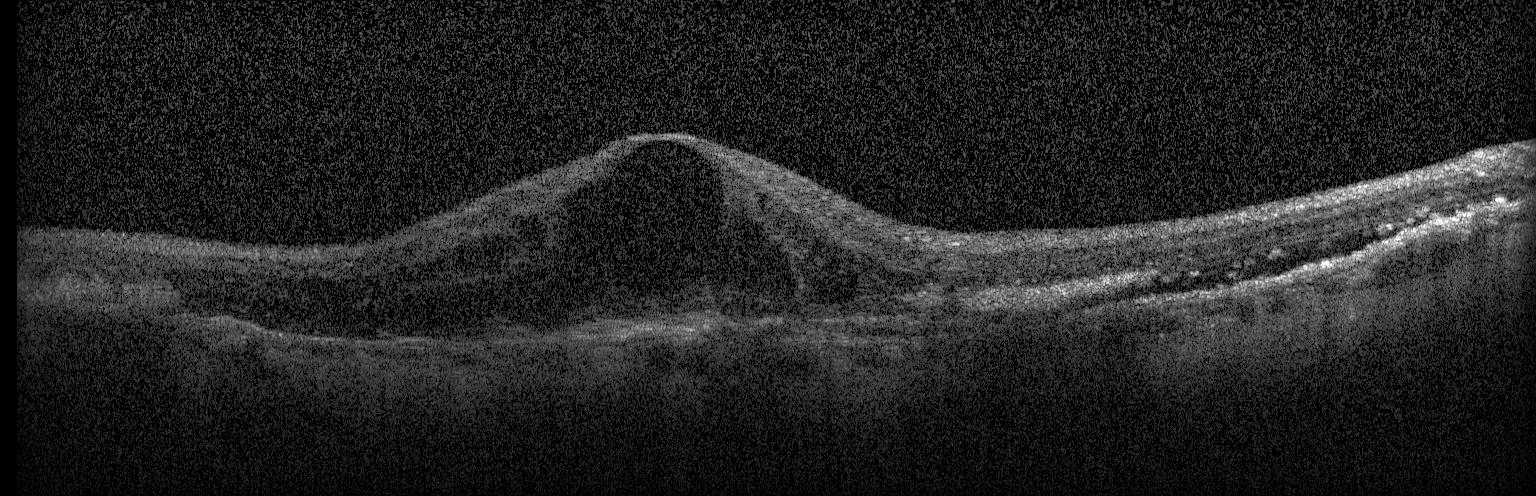 Diagnosis: choroidal neovascularization.